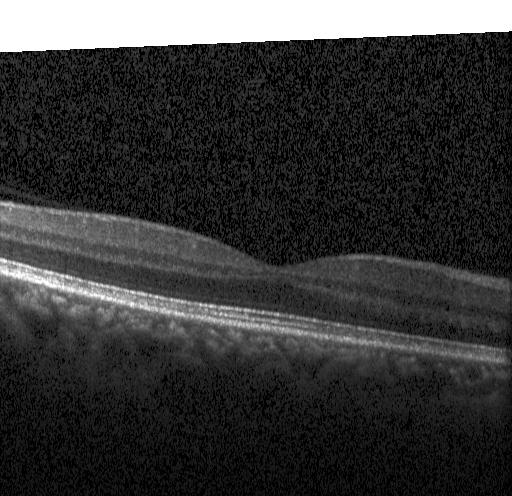 Spectral-domain OCT B-scan: neither choroidal neovascularization, diabetic macular edema, nor drusen.